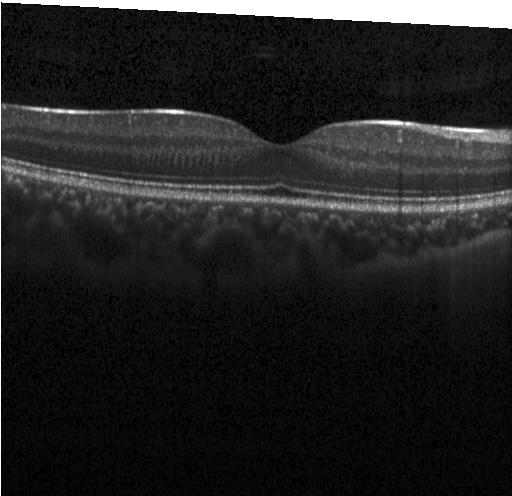 Fovea-centered; instrument: Heidelberg Spectralis; OCT line scan; SD-OCT. Diagnosis: no evidence of choroidal neovascularization, diabetic macular edema, or drusen.